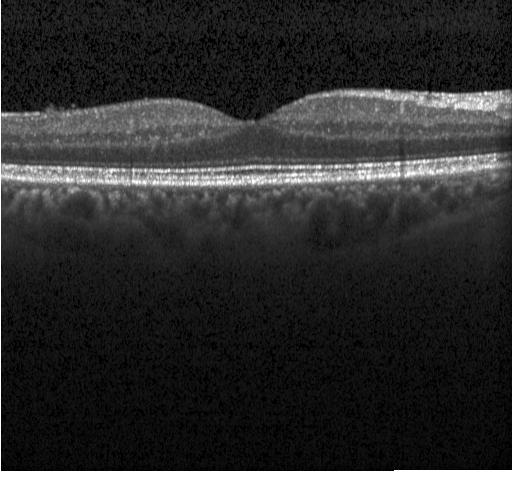

OCT finding: no choroidal neovascularization, diabetic macular edema, or drusen.